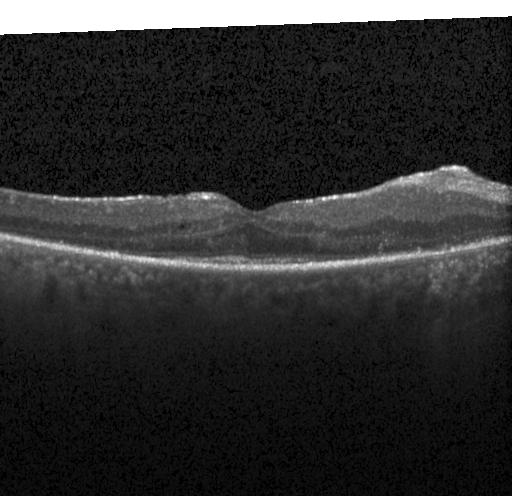

Optical coherence tomography B-scan · spectral-domain OCT · acquired on a Heidelberg Spectralis · centered on the fovea.
This B-scan demonstrates DME.